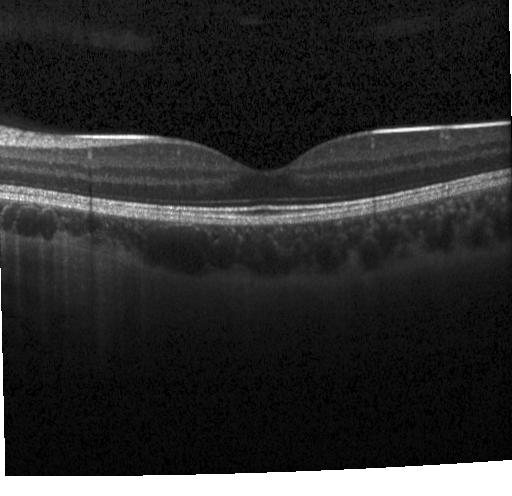 Diagnosis: neither choroidal neovascularization, diabetic macular edema, nor drusen.